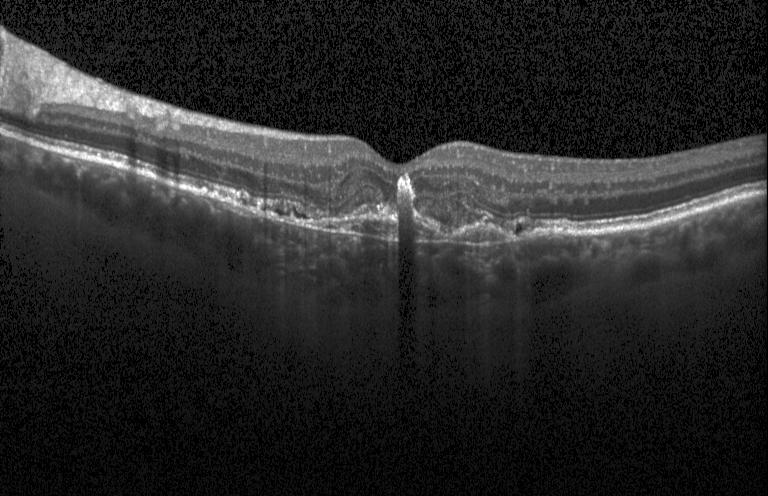 OCT B-scan — Assessment: CNV.